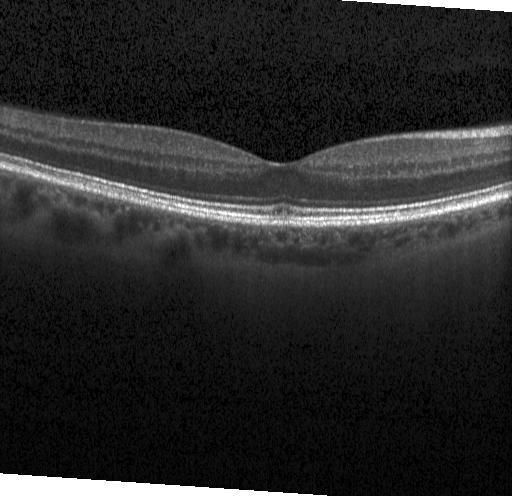

Heidelberg Spectralis OCT system, OCT line scan. Impression: neither CNV, DME, nor drusen.